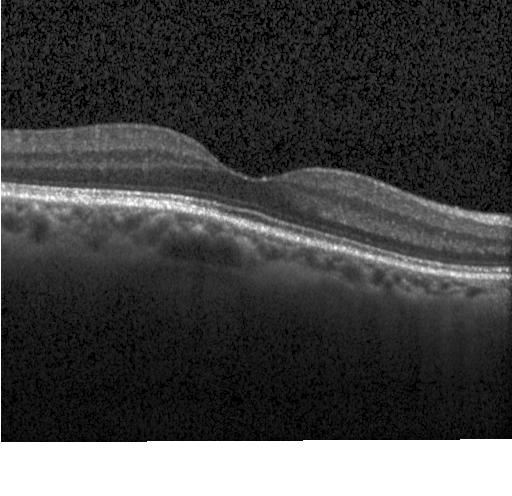
Macular OCT: no choroidal neovascularization, diabetic macular edema, or drusen.